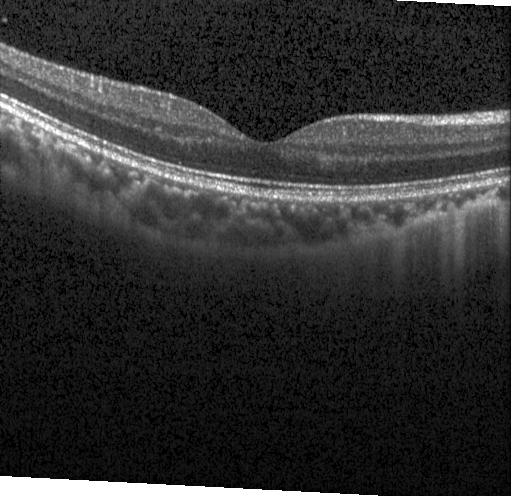
Impression: no CNV, no DME, and no drusen.